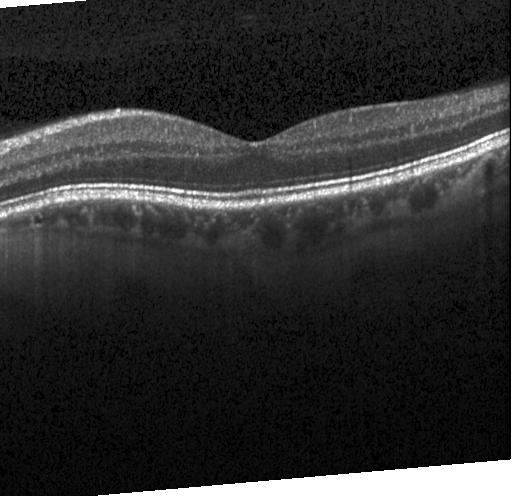 Macular scan; acquired on a Heidelberg Spectralis; optical coherence tomography B-scan; spectral-domain OCT
Impression: no CNV, no DME, and no drusen.